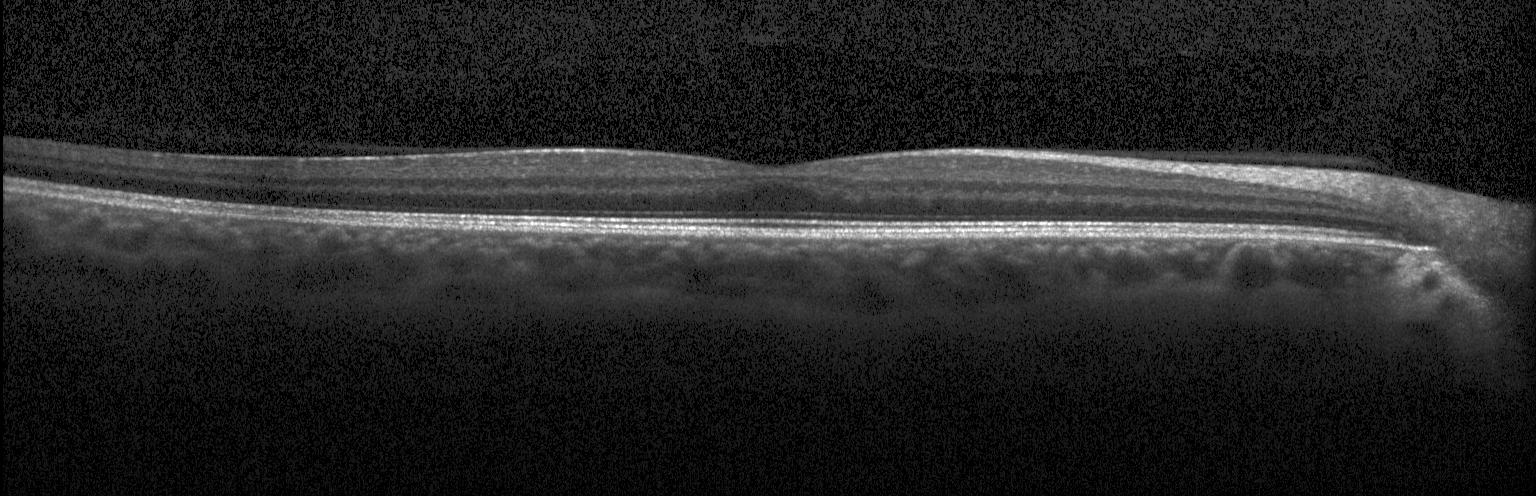 Dx: no choroidal neovascularization, no diabetic macular edema, and no drusen.